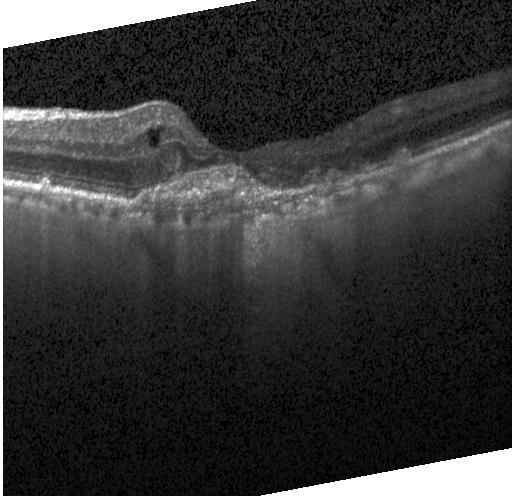

Diagnosis: a choroidal neovascular membrane.